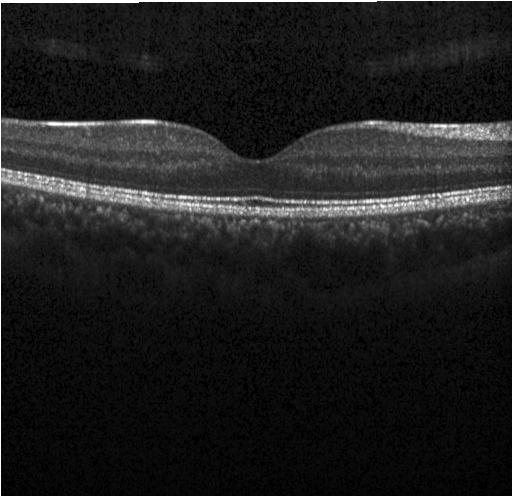

Spectral-domain OCT B-scan: no CNV, DME, or drusen.